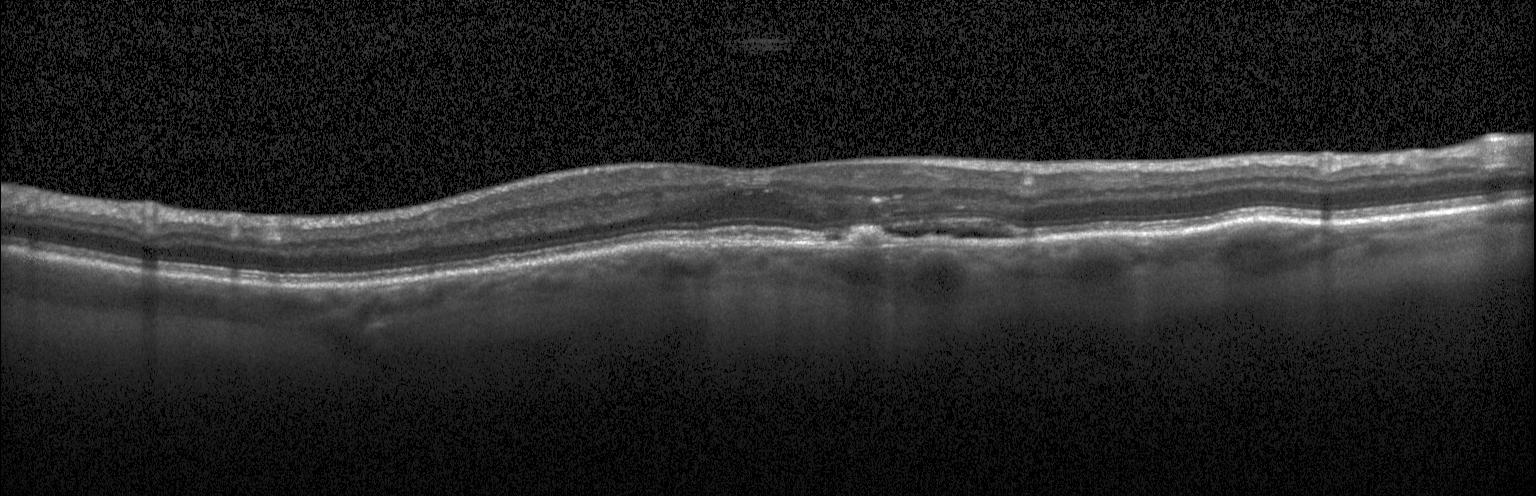
Retinal OCT B-scan · SD-OCT · centered on the fovea · acquired on a Heidelberg Spectralis
Diagnosis: CNV.